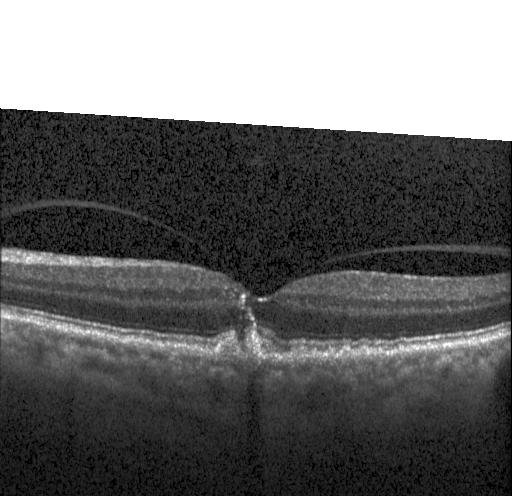

Optical coherence tomography B-scan; SD-OCT; fovea-centered; Heidelberg Spectralis.
Finding: sub-RPE drusenoid deposits.